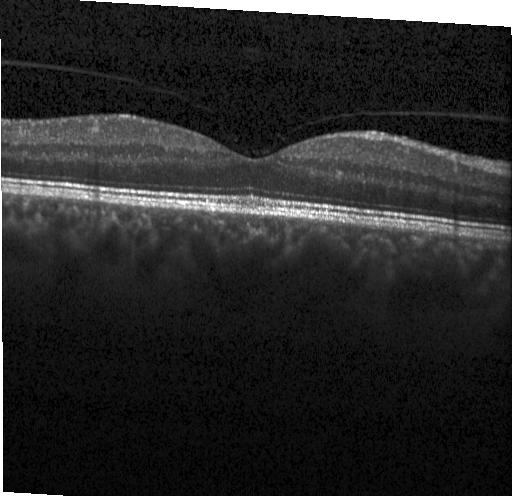 Fovea-centered · retinal OCT B-scan
Dx: no choroidal neovascularization, diabetic macular edema, or drusen.